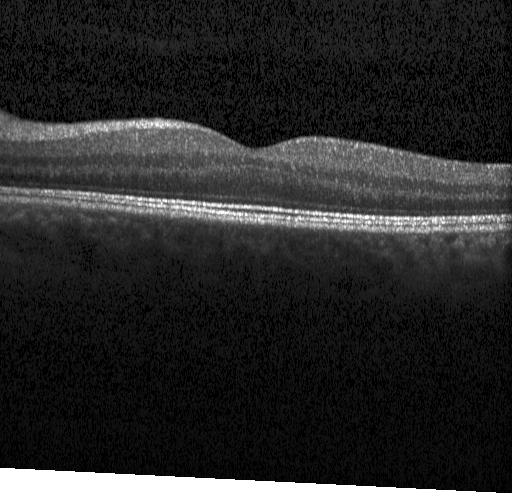
OCT B-scan, Heidelberg Spectralis.
This B-scan demonstrates neither CNV, DME, nor drusen.